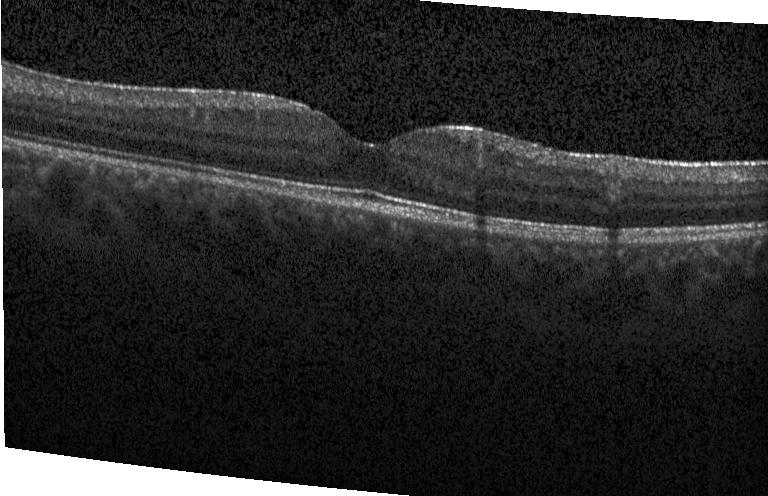
OCT B-scan, SD-OCT. Impression: no choroidal neovascularization, no diabetic macular edema, and no drusen.